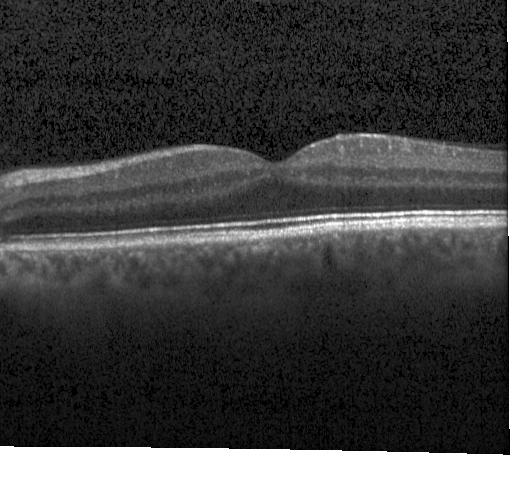
Impression: neither choroidal neovascularization, diabetic macular edema, nor drusen.